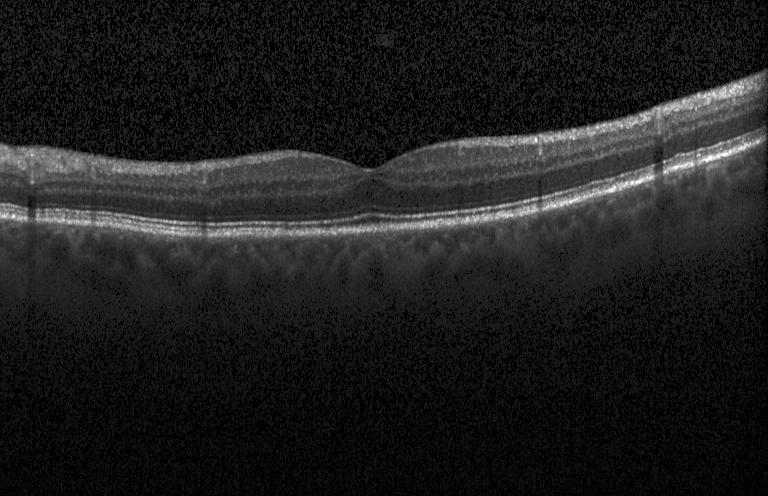
Impression: neither choroidal neovascularization, diabetic macular edema, nor drusen.